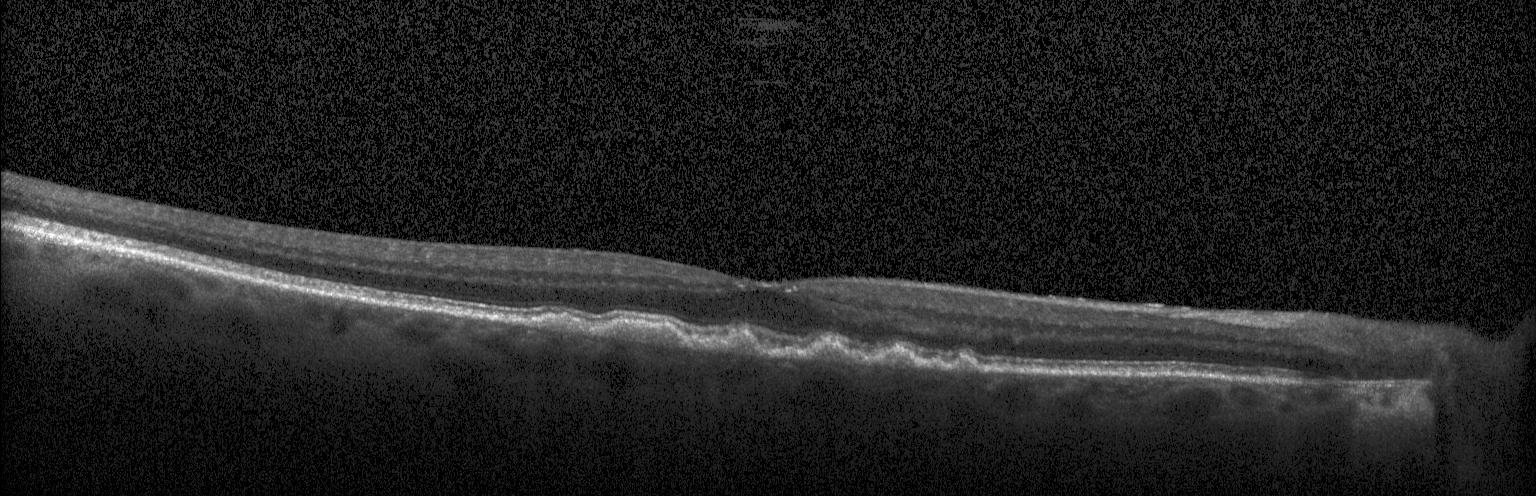
OCT finding: sub-RPE drusenoid deposits.